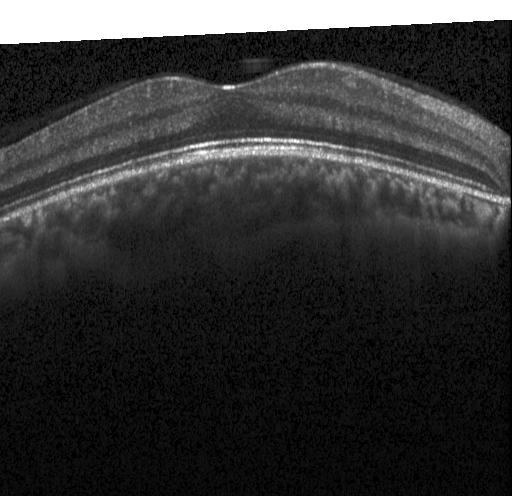

Optical coherence tomography B-scan. Through the macula. Finding: neither CNV, DME, nor drusen.